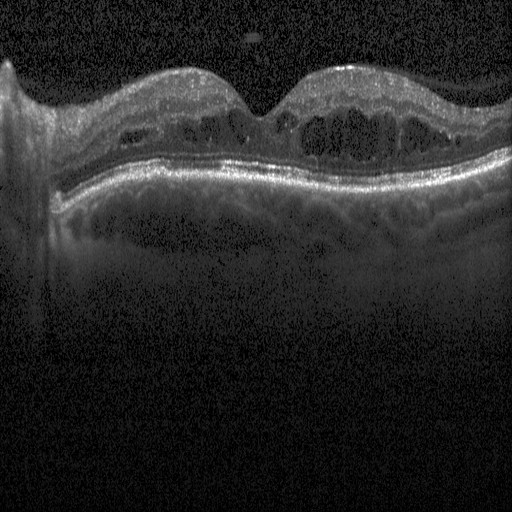
Diagnosis: DME.